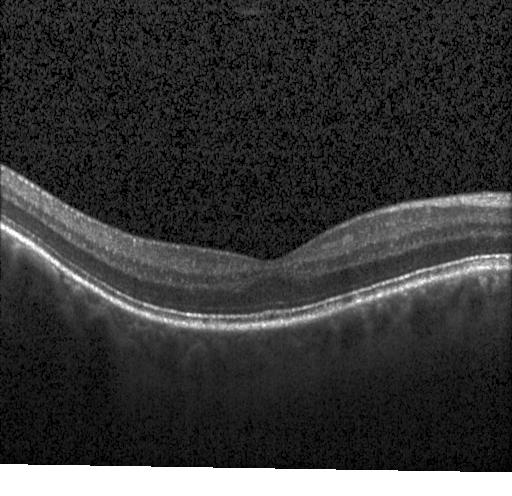

Finding: no choroidal neovascularization, diabetic macular edema, or drusen.